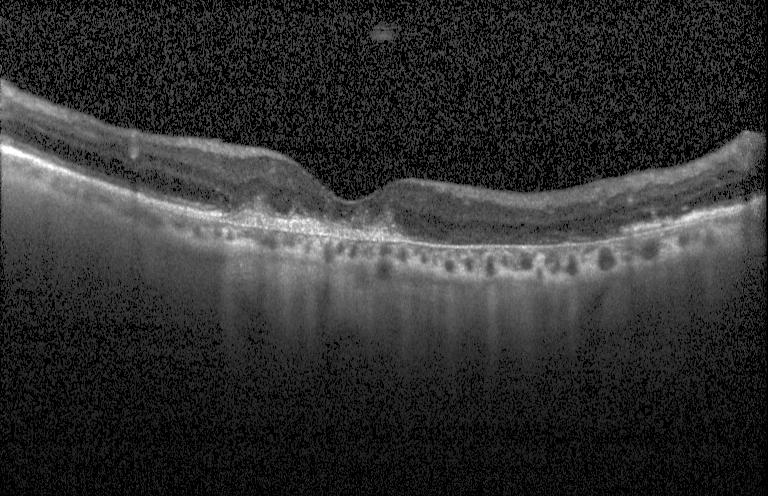 OCT scan showing a choroidal neovascular membrane.